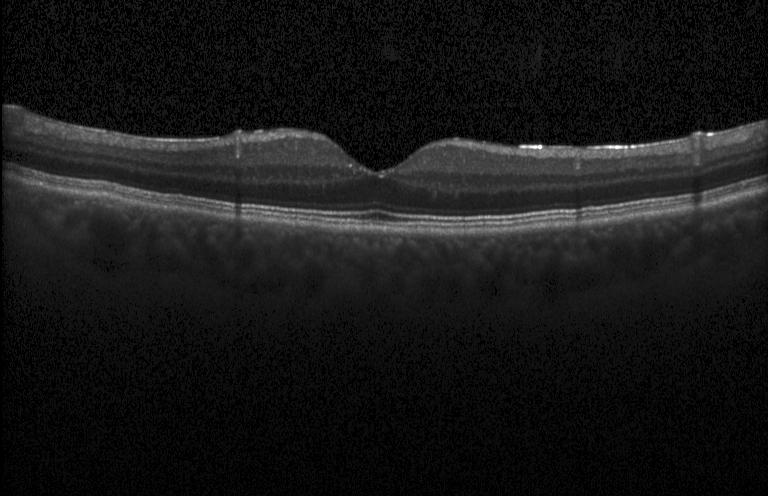
Assessment: neither CNV, DME, nor drusen.